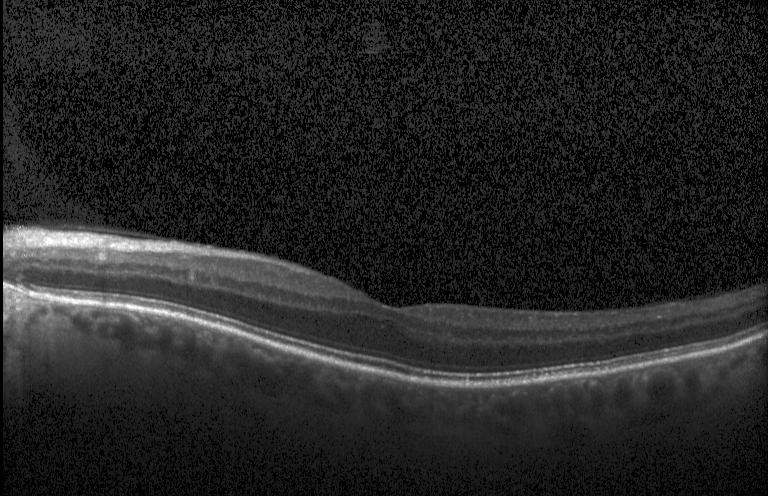
Optical coherence tomography scan, through the macula, spectral-domain optical coherence tomography.
Diagnosis: no choroidal neovascularization, no diabetic macular edema, and no drusen.